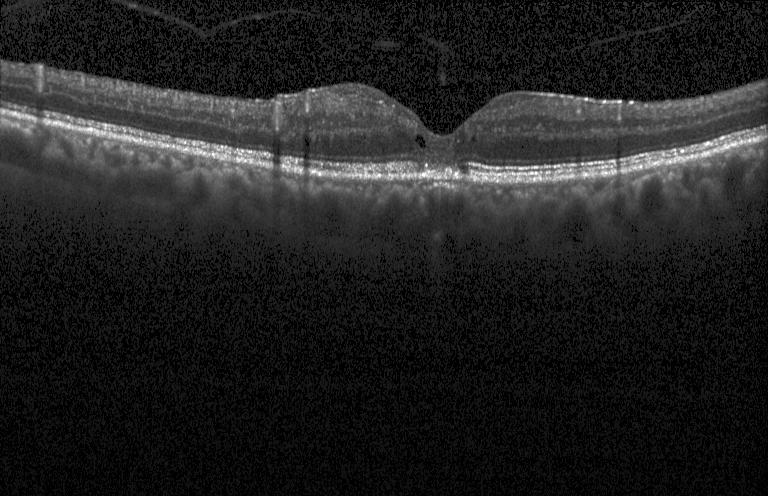 Spectral-domain optical coherence tomography · horizontal scan through the fovea · OCT line scan.
Assessment: diabetic macular edema (DME).